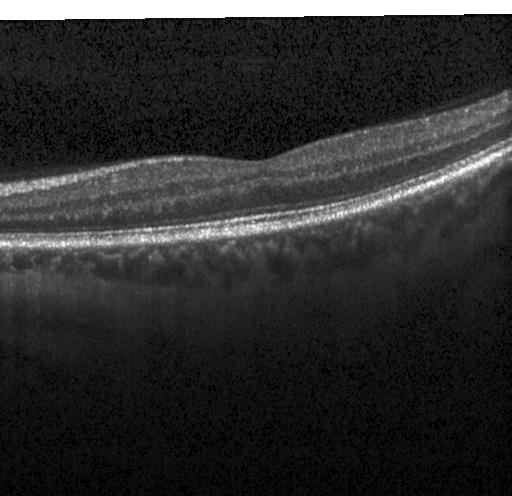

Fovea-centered, spectral-domain OCT, acquired on a Heidelberg Spectralis, optical coherence tomography B-scan — Macular OCT: no evidence of choroidal neovascularization, diabetic macular edema, or drusen.